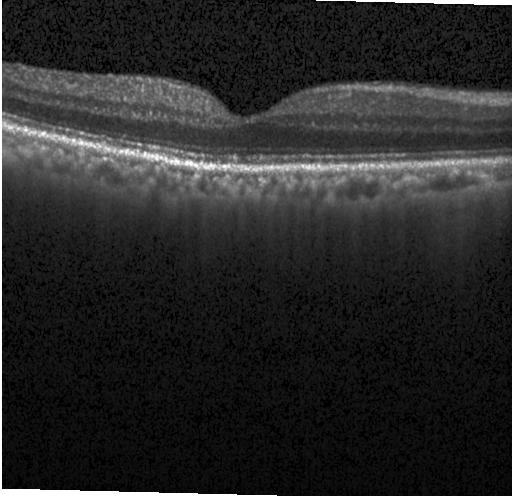 OCT finding: neither CNV, DME, nor drusen.